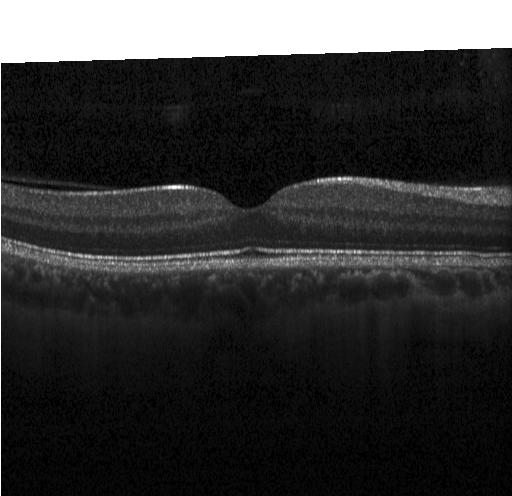 Retinal OCT B-scan
Diagnosis: no choroidal neovascularization, no diabetic macular edema, and no drusen.